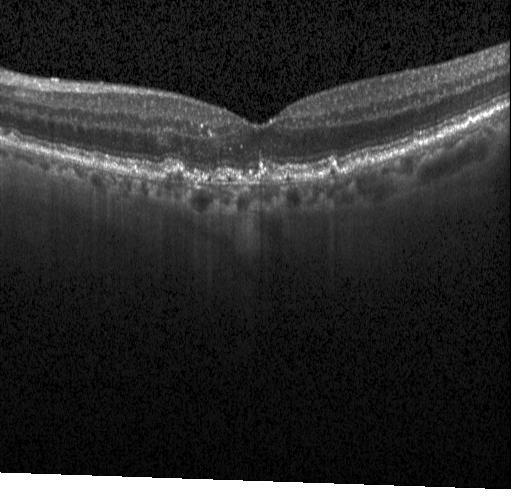
Diagnosis: multiple drusen.